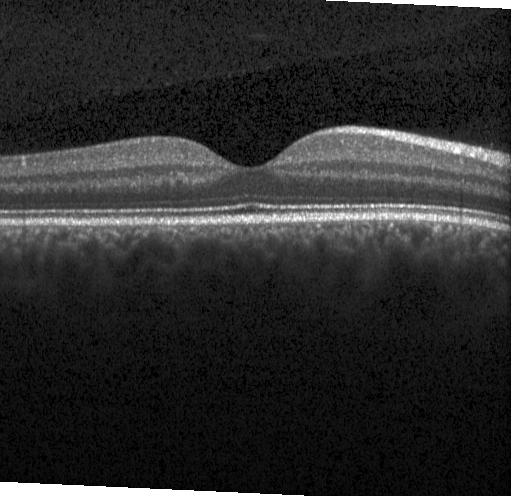
Spectral-domain optical coherence tomography; OCT B-scan; acquired on a Heidelberg Spectralis; macular scan — OCT finding: no choroidal neovascularization, diabetic macular edema, or drusen.